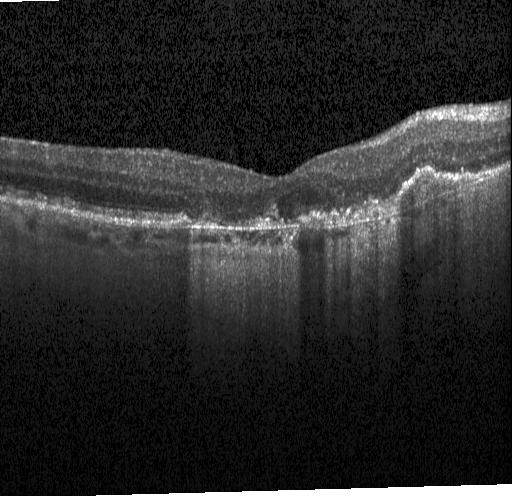 Instrument: Heidelberg Spectralis. Retinal OCT cross-section. SD-OCT. Fovea-centered — Assessment: choroidal neovascularization.